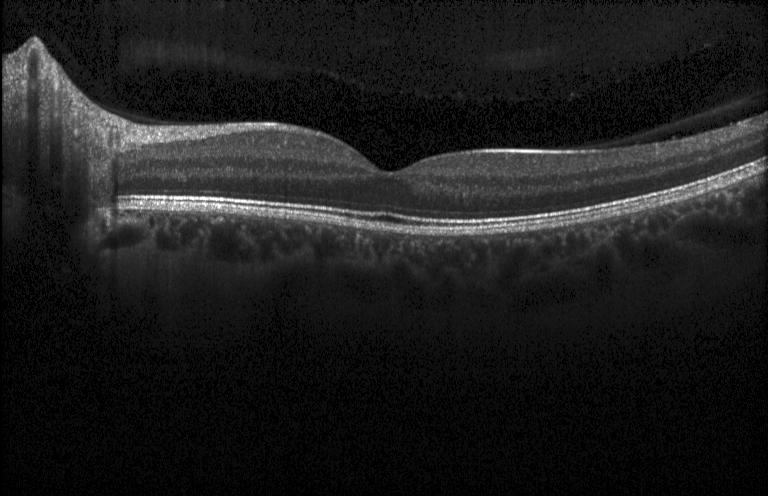

OCT line scan; spectral-domain OCT; fovea-centered; instrument: Heidelberg Spectralis.
Impression: no choroidal neovascularization, diabetic macular edema, or drusen.